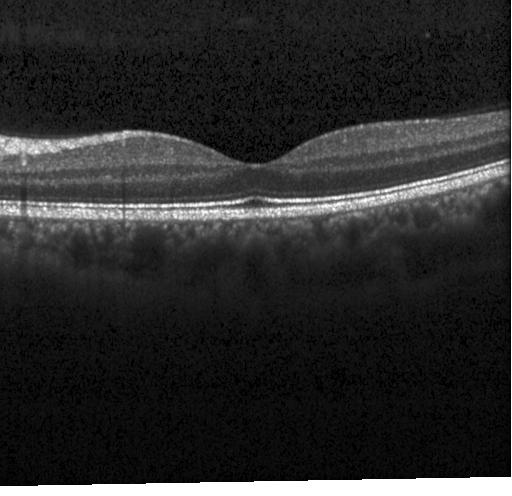

Retinal OCT B-scan
Dx: no CNV, no DME, and no drusen.